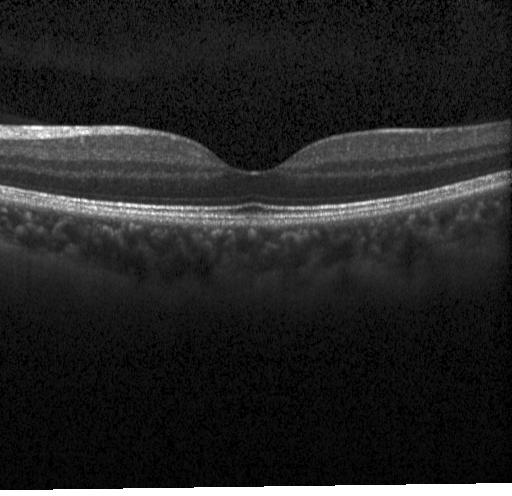 Finding: no evidence of CNV, DME, or drusen.